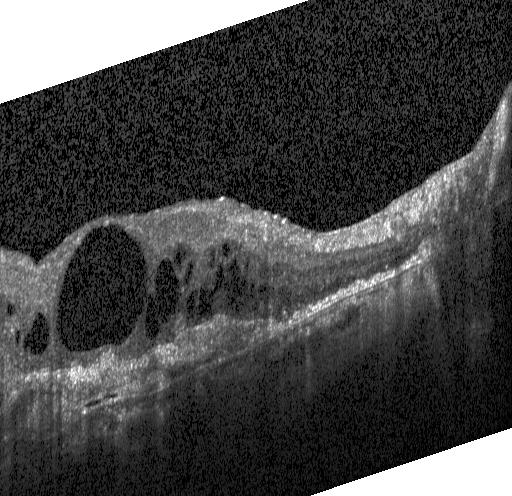 Through the macula; retinal OCT cross-section.
Diagnosis: CNV.